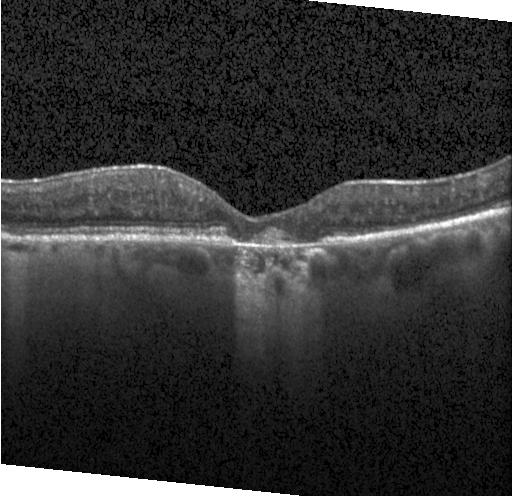

Optical coherence tomography B-scan; SD-OCT; instrument: Heidelberg Spectralis; centered on the fovea. Assessment: a choroidal neovascular membrane.